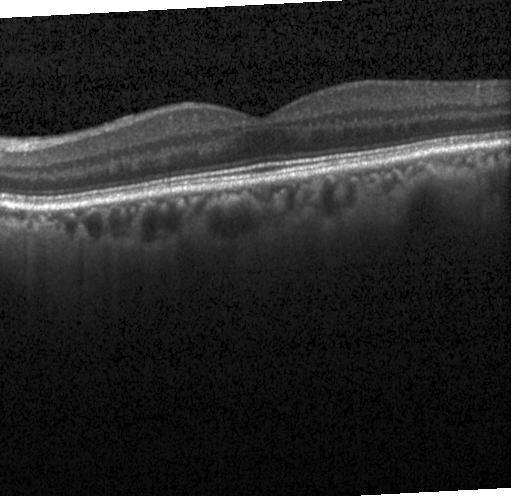 Spectral-domain optical coherence tomography. OCT B-scan. Acquired on a Heidelberg Spectralis.
Diagnosis: neither choroidal neovascularization, diabetic macular edema, nor drusen.